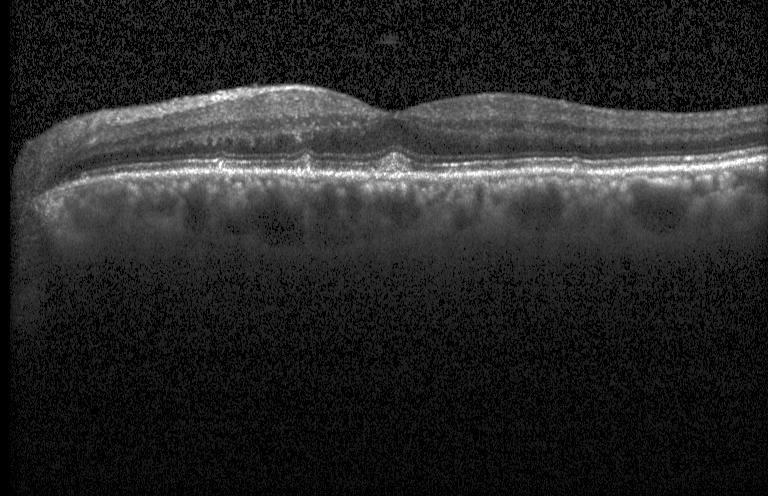 Spectral-domain OCT, optical coherence tomography scan, acquired on a Heidelberg Spectralis. Finding: sub-RPE drusenoid deposits.